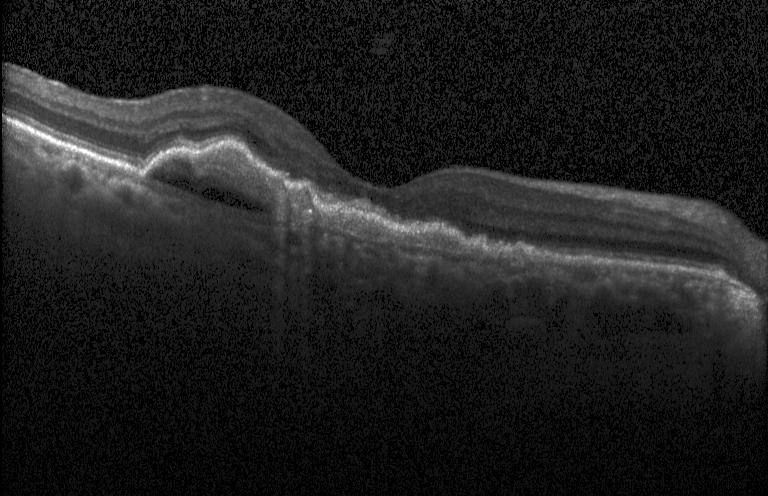

Spectral-domain optical coherence tomography; optical coherence tomography scan
Choroidal neovascularization (CNV).